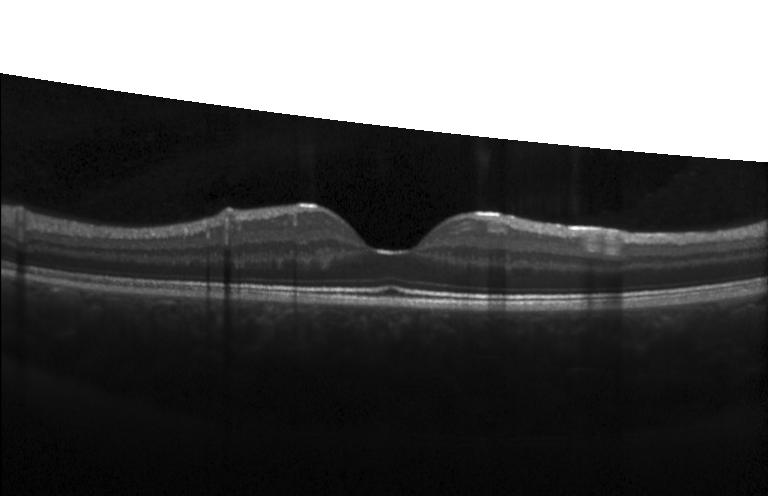
Centered on the fovea · retinal OCT B-scan
This B-scan demonstrates neither CNV, DME, nor drusen.